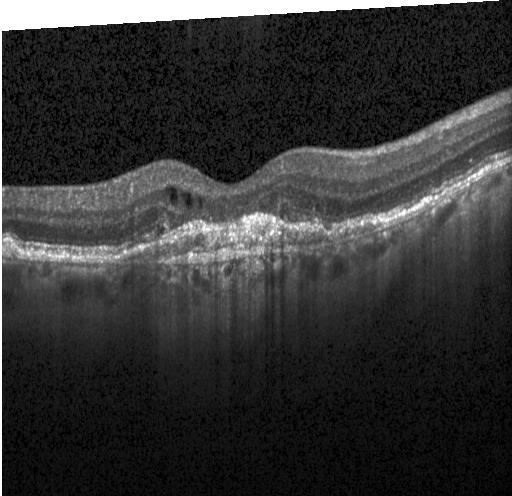

Optical coherence tomography scan; spectral-domain OCT; acquired on a Heidelberg Spectralis
A choroidal neovascular membrane.